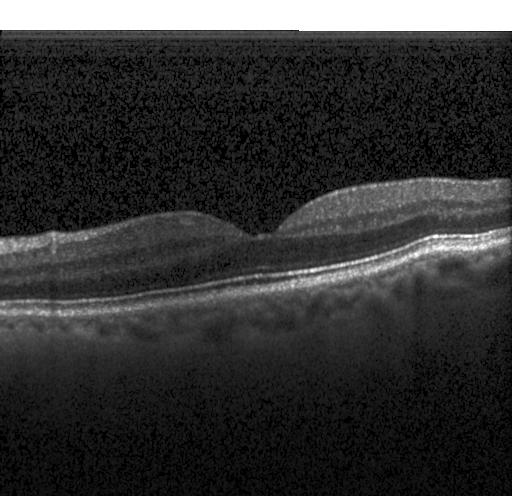
Retinal OCT B-scan · horizontal scan through the fovea · acquired on a Heidelberg Spectralis · spectral-domain OCT — Impression: no choroidal neovascularization, no diabetic macular edema, and no drusen.